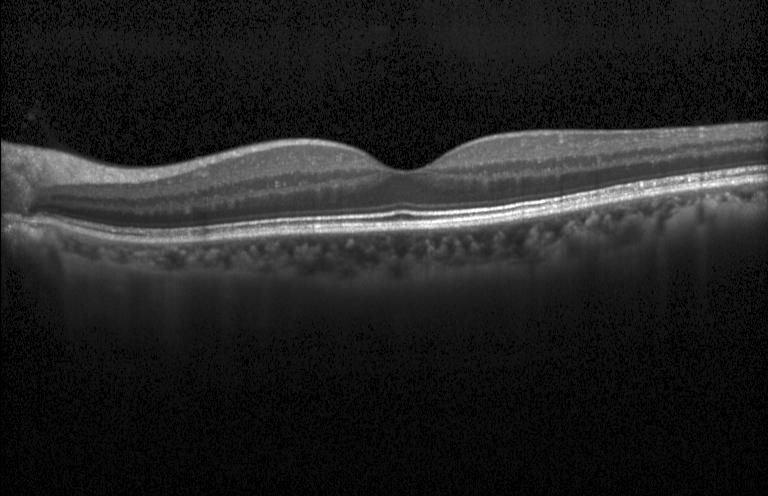

Spectral-domain OCT. Optical coherence tomography scan. Centered on the fovea. Heidelberg Spectralis OCT system.
Impression: no evidence of CNV, DME, or drusen.